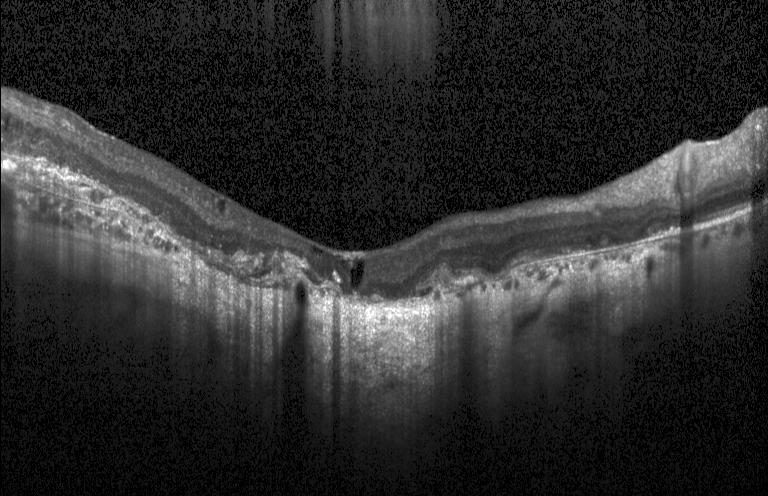
OCT line scan.
Impression: CNV.